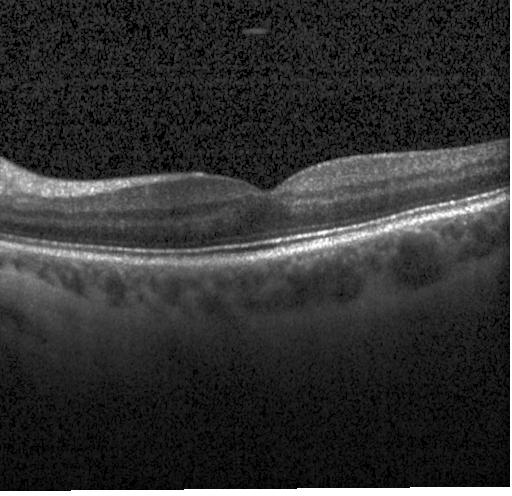 The scan shows no evidence of CNV, DME, or drusen.